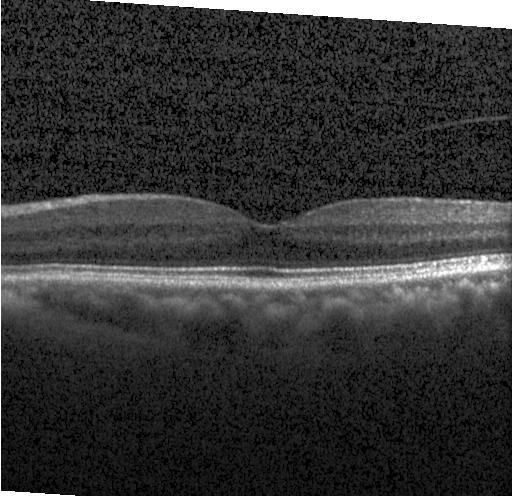

Diagnosis: no evidence of choroidal neovascularization, diabetic macular edema, or drusen.